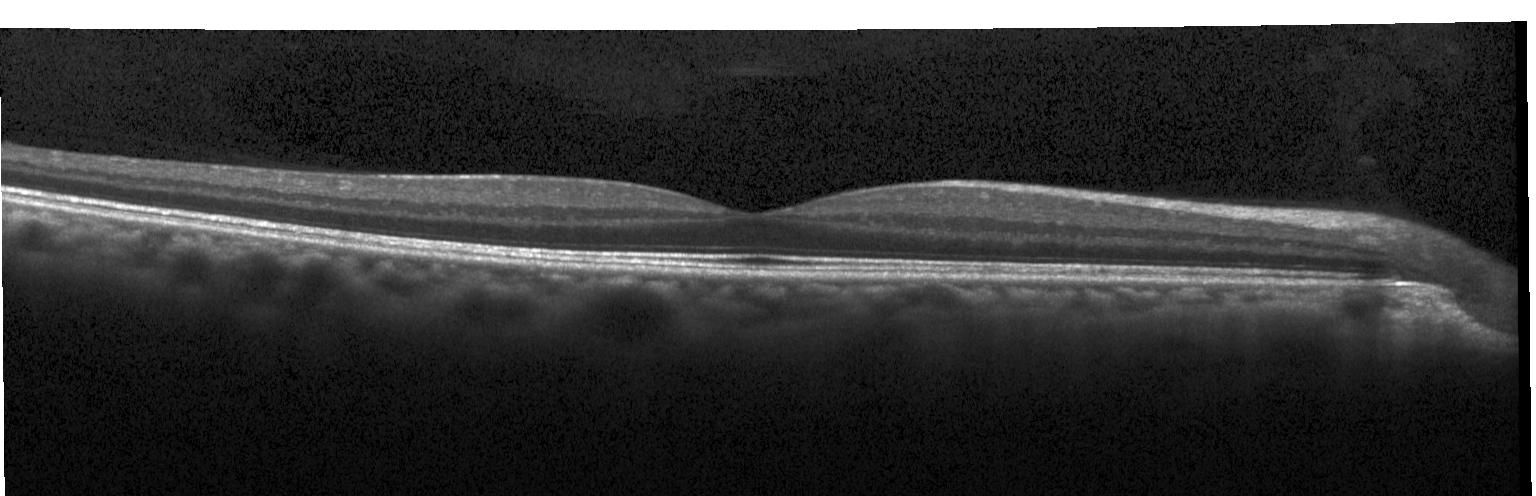

OCT B-scan — Neither CNV, DME, nor drusen.